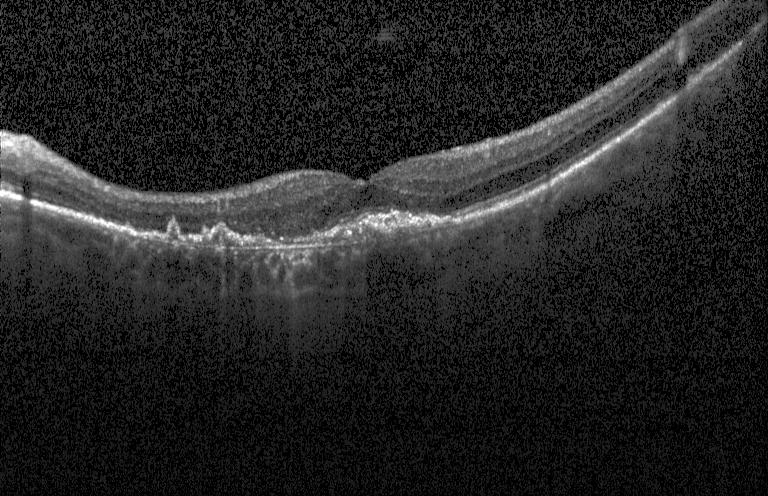 Dx: choroidal neovascularization.